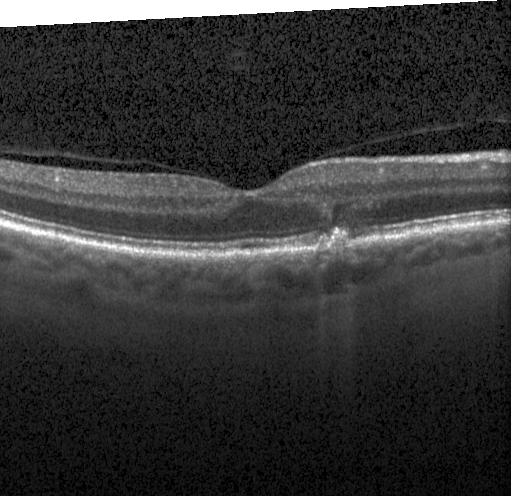

Heidelberg Spectralis OCT system · OCT B-scan · spectral-domain OCT · fovea-centered — Assessment: drusen.